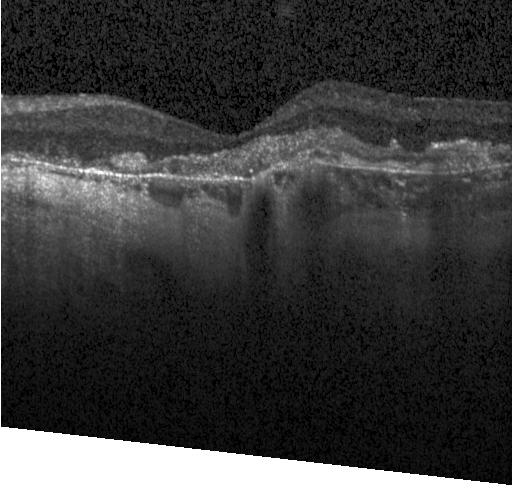 Spectral-domain OCT. Instrument: Heidelberg Spectralis. Macular scan. Optical coherence tomography B-scan.
Finding: a choroidal neovascular membrane.